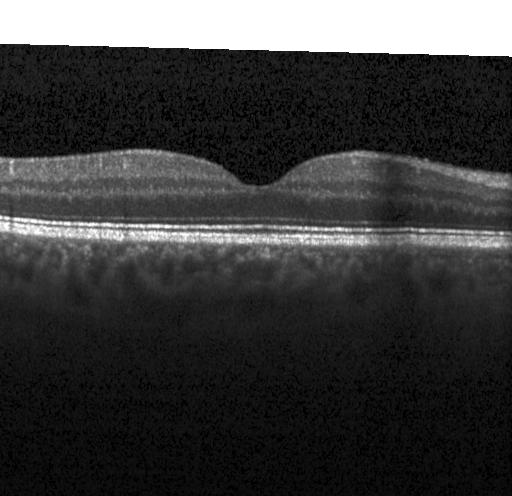

Dx: neither CNV, DME, nor drusen.